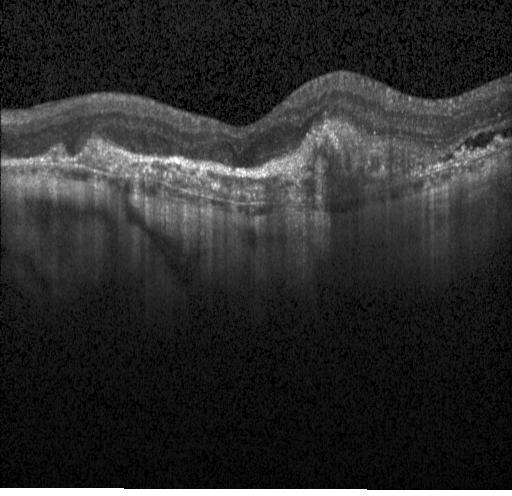

Retinal OCT B-scan
Diagnosis: choroidal neovascularization.